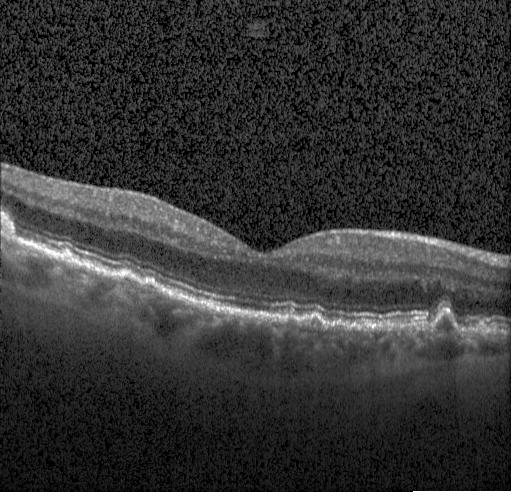

Finding: multiple drusen.